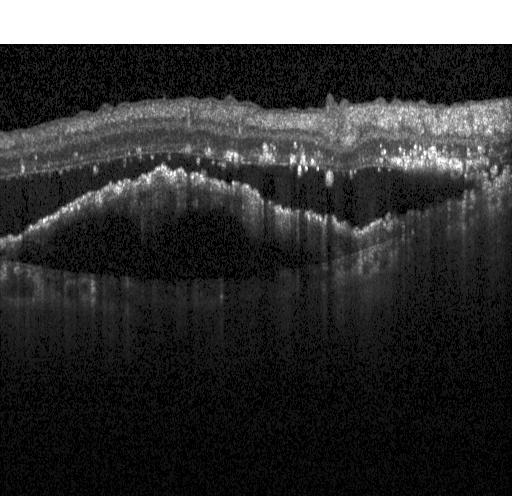
Heidelberg Spectralis OCT system. Retinal OCT cross-section — Macular OCT: a choroidal neovascular membrane.